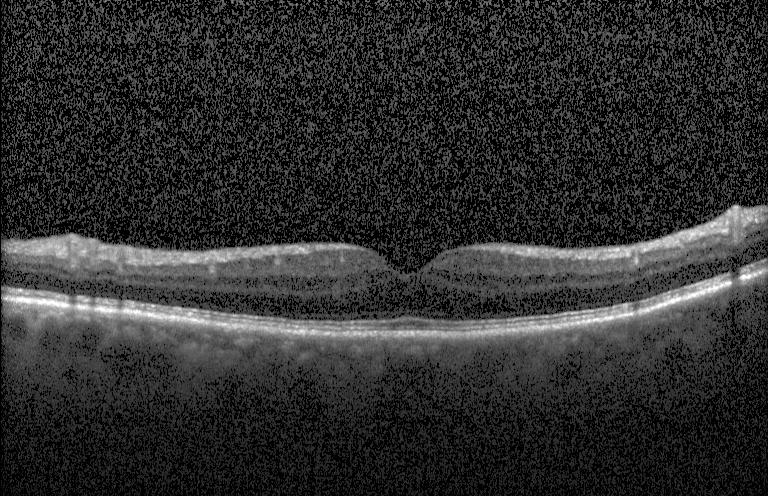

Optical coherence tomography B-scan. Macular OCT: neither CNV, DME, nor drusen.